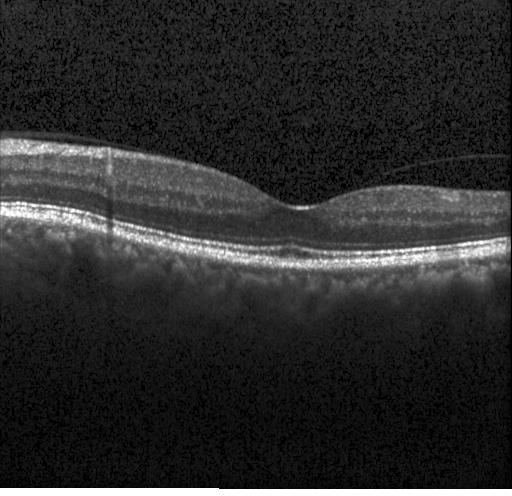 Spectral-domain OCT, through the macula, retinal OCT cross-section — Assessment: no choroidal neovascularization, diabetic macular edema, or drusen.